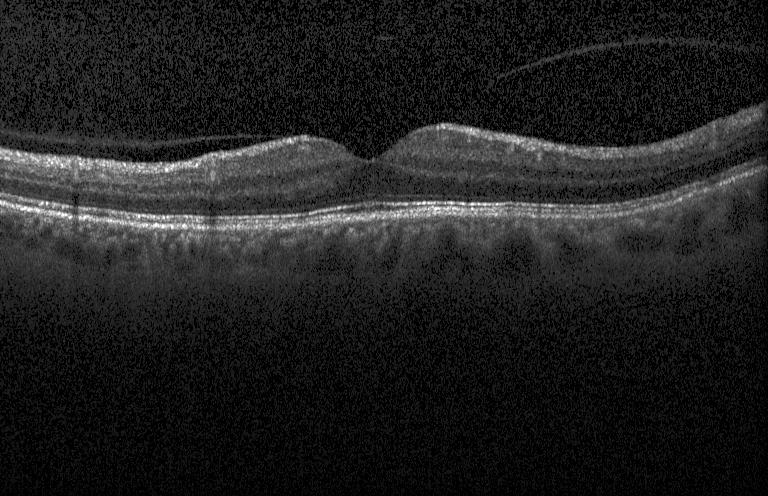
Optical coherence tomography B-scan. Spectral-domain OCT — This B-scan demonstrates no evidence of choroidal neovascularization, diabetic macular edema, or drusen.